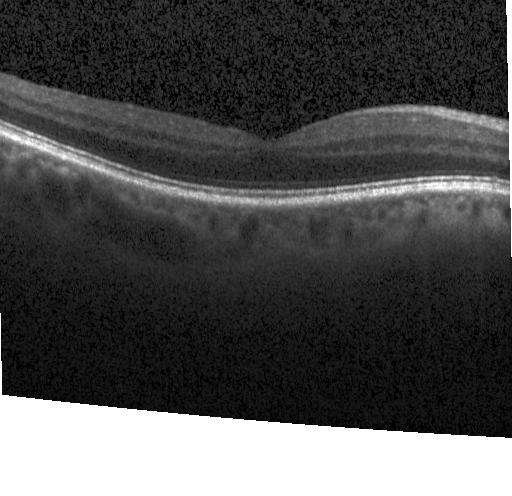

Heidelberg Spectralis OCT system. Spectral-domain OCT. Fovea-centered. Optical coherence tomography B-scan. Impression: no choroidal neovascularization, no diabetic macular edema, and no drusen.